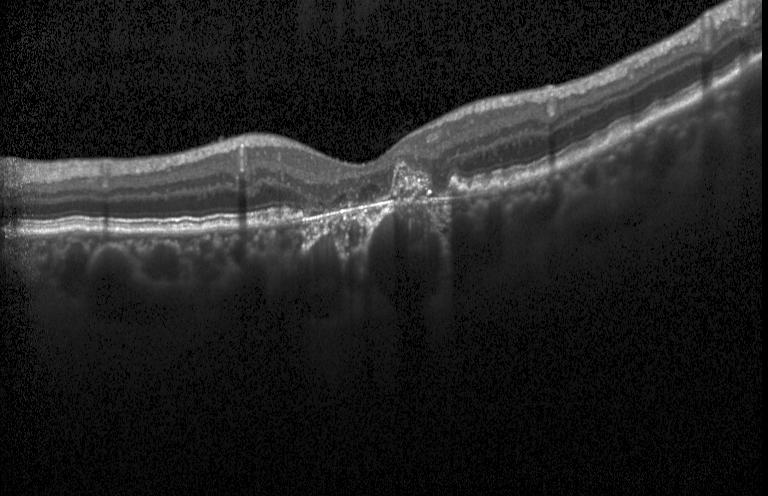
SD-OCT · fovea-centered · OCT line scan · Heidelberg Spectralis OCT system
A choroidal neovascular membrane.